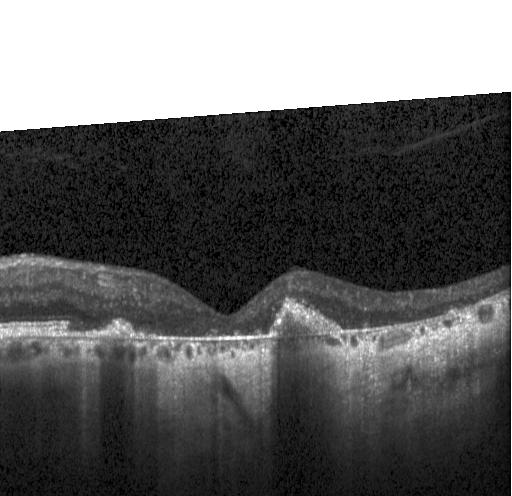

Optical coherence tomography B-scan; instrument: Heidelberg Spectralis. This B-scan demonstrates choroidal neovascularization (CNV).